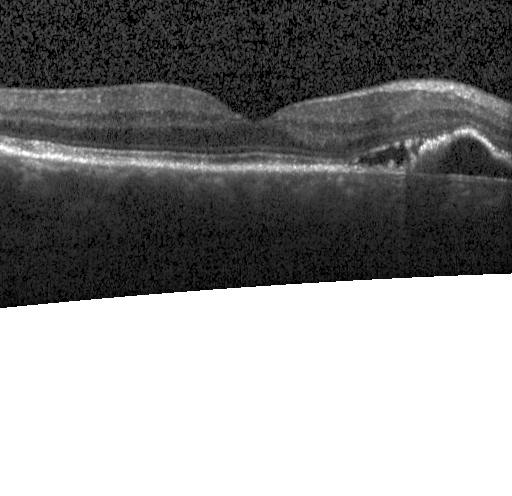 Macular OCT: a choroidal neovascular membrane.